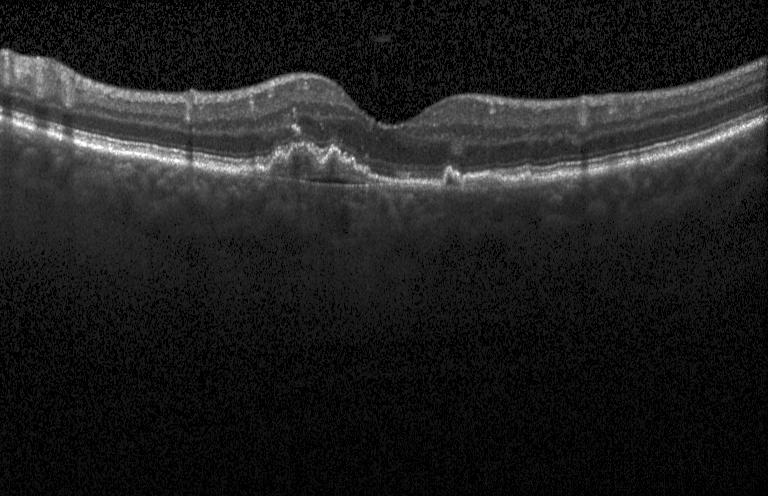
Macular OCT: CNV.